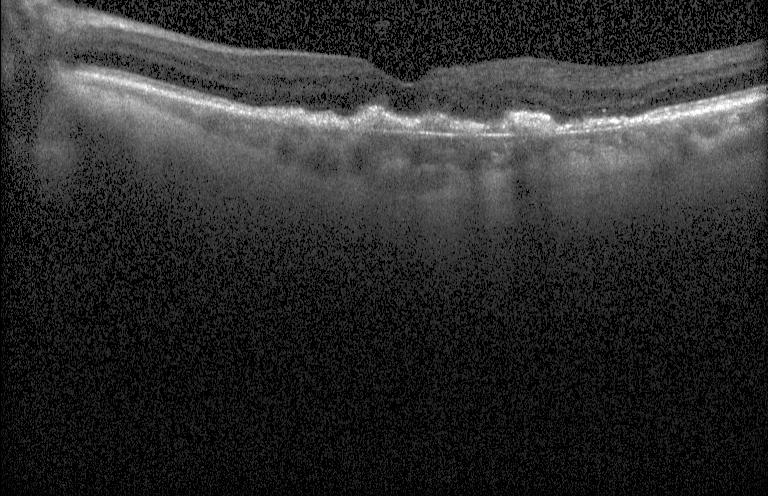 Retinal OCT B-scan.
OCT finding: a choroidal neovascular membrane.